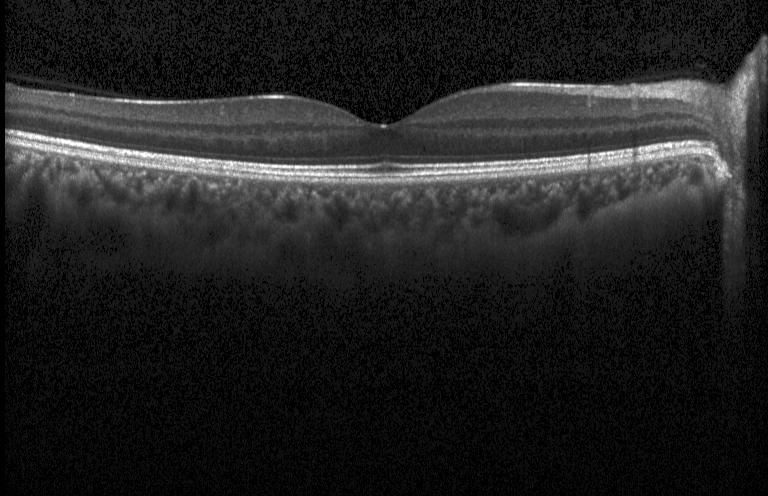 Finding: no choroidal neovascularization, diabetic macular edema, or drusen.